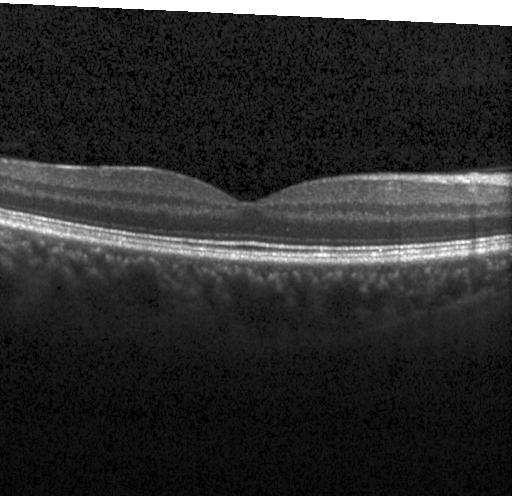 Dx: neither choroidal neovascularization, diabetic macular edema, nor drusen.